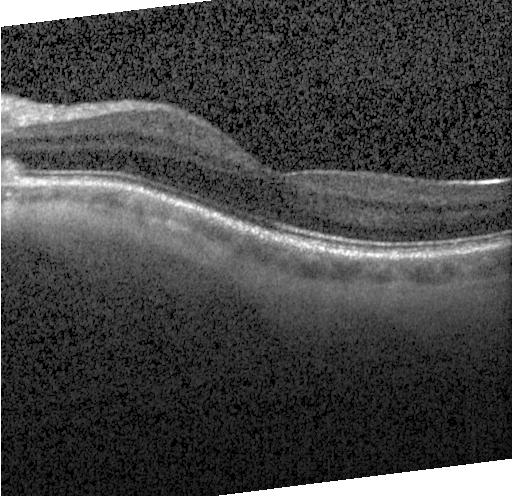 Optical coherence tomography B-scan; spectral-domain optical coherence tomography; horizontal scan through the fovea
Impression: sub-RPE drusenoid deposits.